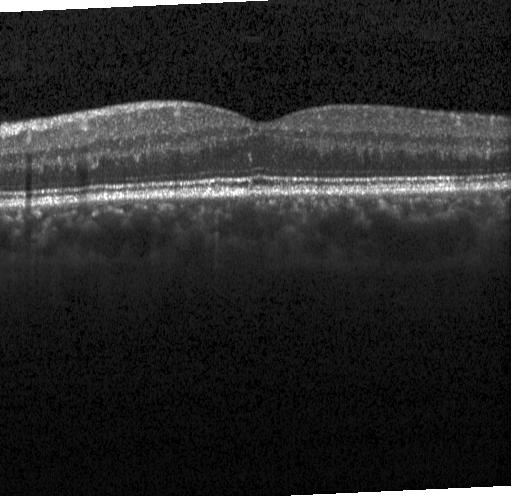
Macular scan; optical coherence tomography B-scan.
This B-scan demonstrates neither choroidal neovascularization, diabetic macular edema, nor drusen.